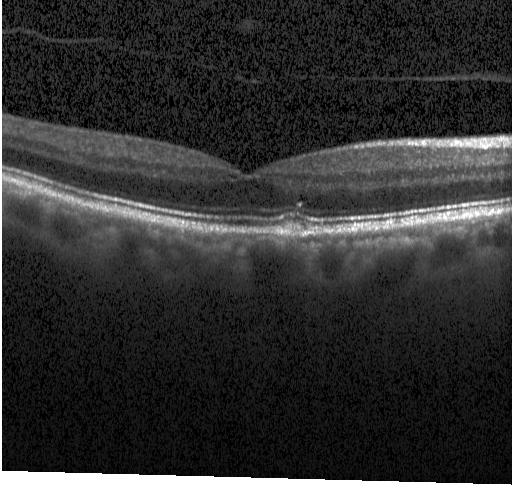

Optical coherence tomography scan. This B-scan demonstrates sub-RPE drusenoid deposits.